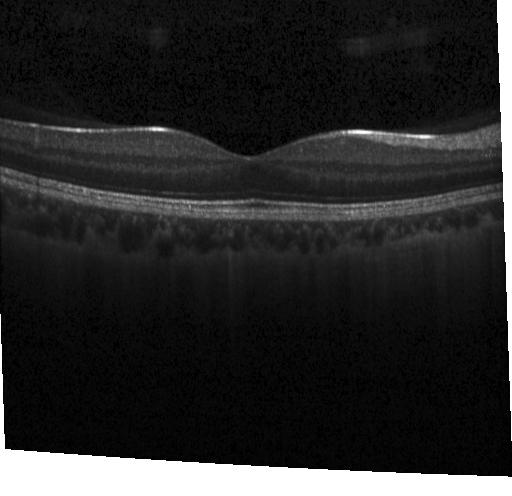 OCT finding: no choroidal neovascularization, no diabetic macular edema, and no drusen.